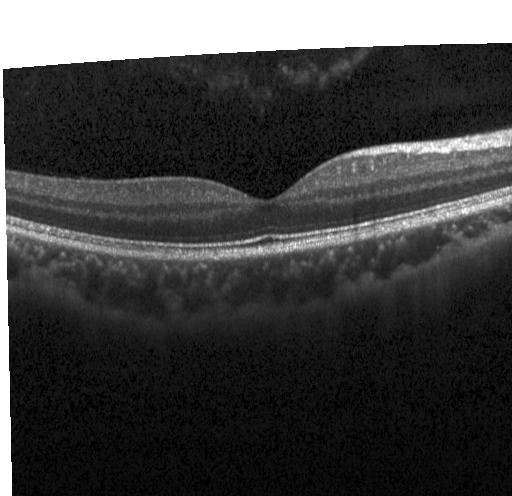 Retinal OCT B-scan — Impression: neither CNV, DME, nor drusen.